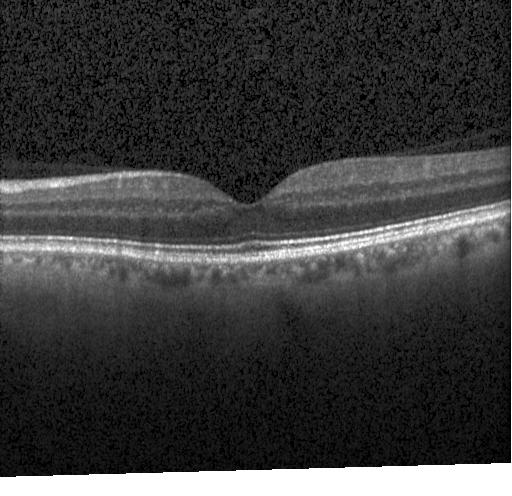
Spectral-domain OCT B-scan: no evidence of CNV, DME, or drusen.